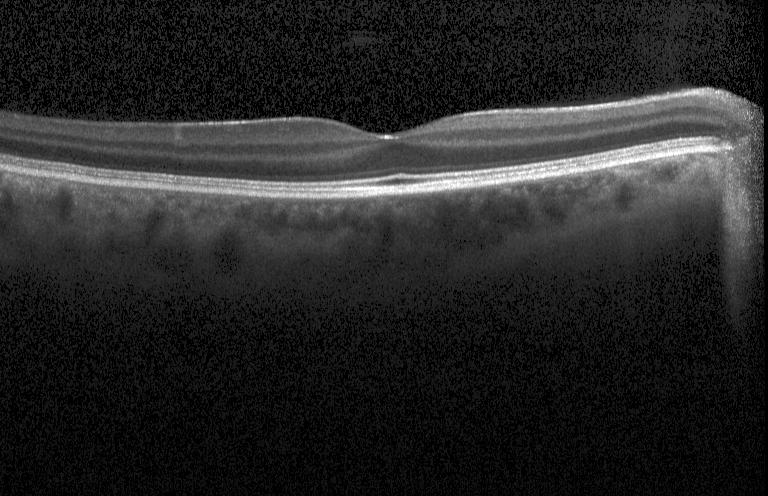 Through the macula. OCT B-scan. SD-OCT
The scan shows neither choroidal neovascularization, diabetic macular edema, nor drusen.